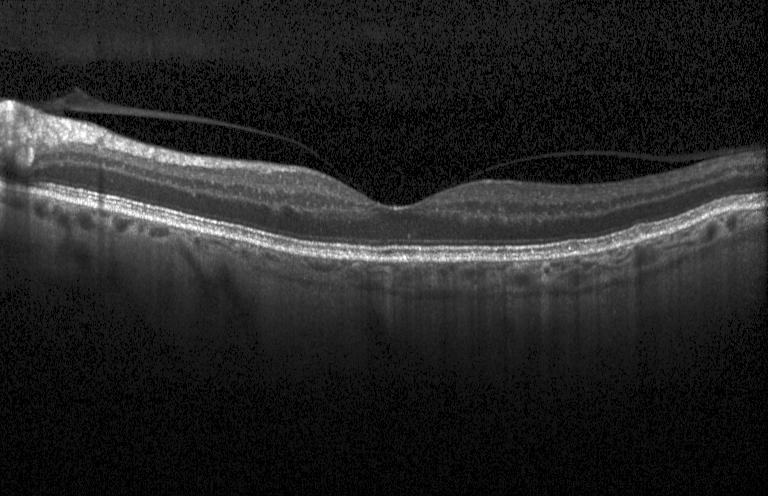

Horizontal scan through the fovea. Heidelberg Spectralis. Retinal OCT cross-section. SD-OCT — Finding: no choroidal neovascularization, diabetic macular edema, or drusen.